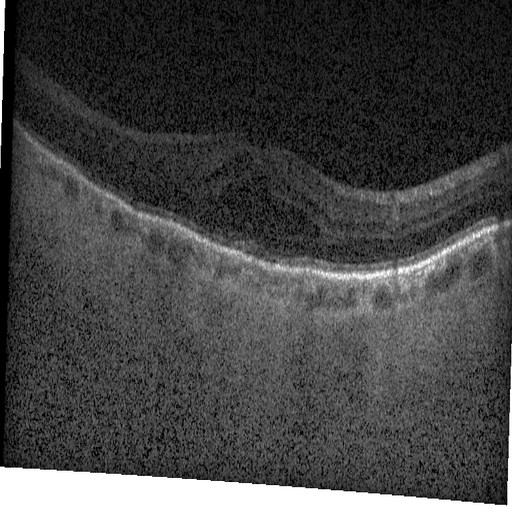
Instrument: Heidelberg Spectralis · spectral-domain OCT · optical coherence tomography scan · through the macula — This B-scan demonstrates DME.